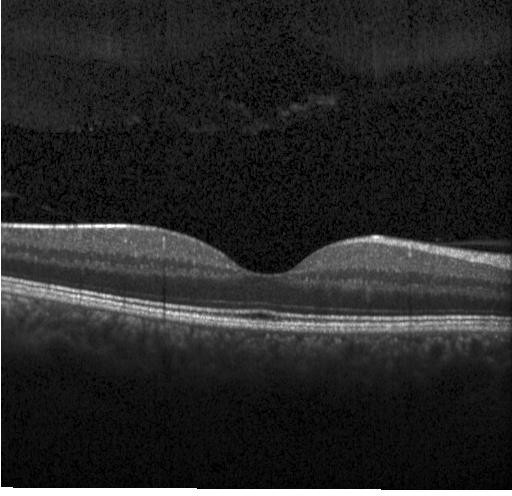 SD-OCT. Retinal OCT cross-section. Finding: no choroidal neovascularization, no diabetic macular edema, and no drusen.